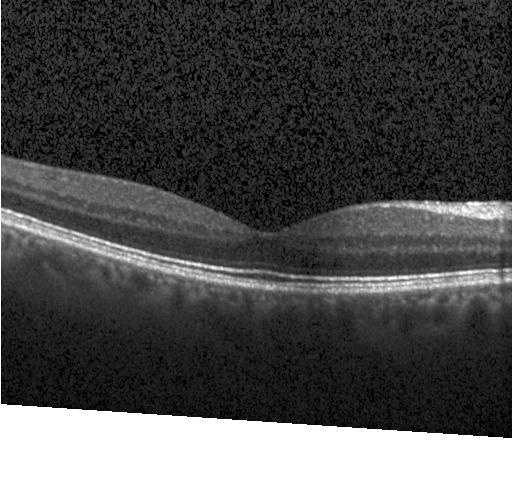 Diagnosis: no evidence of choroidal neovascularization, diabetic macular edema, or drusen.